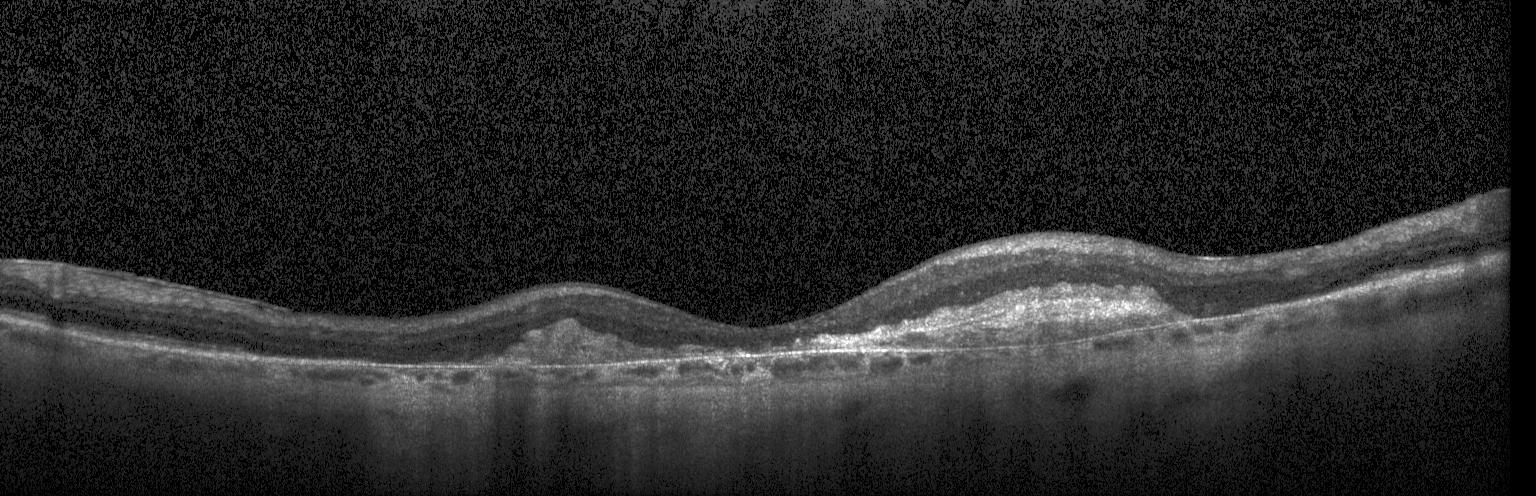 Retinal OCT cross-section. Diagnosis: a choroidal neovascular membrane.